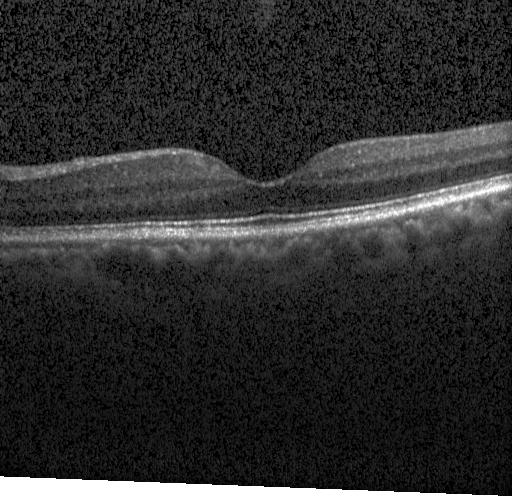

Diagnosis: no choroidal neovascularization, diabetic macular edema, or drusen.